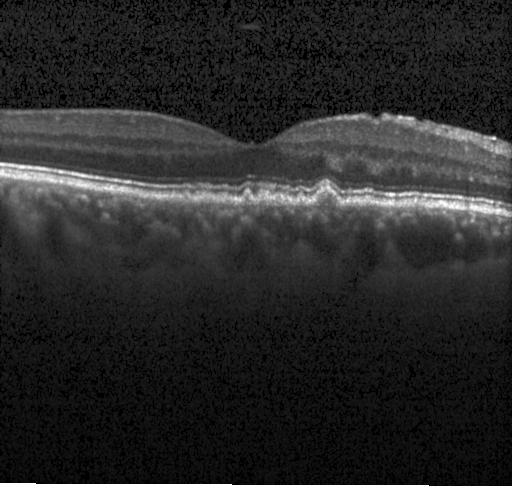

OCT scan showing drusen.